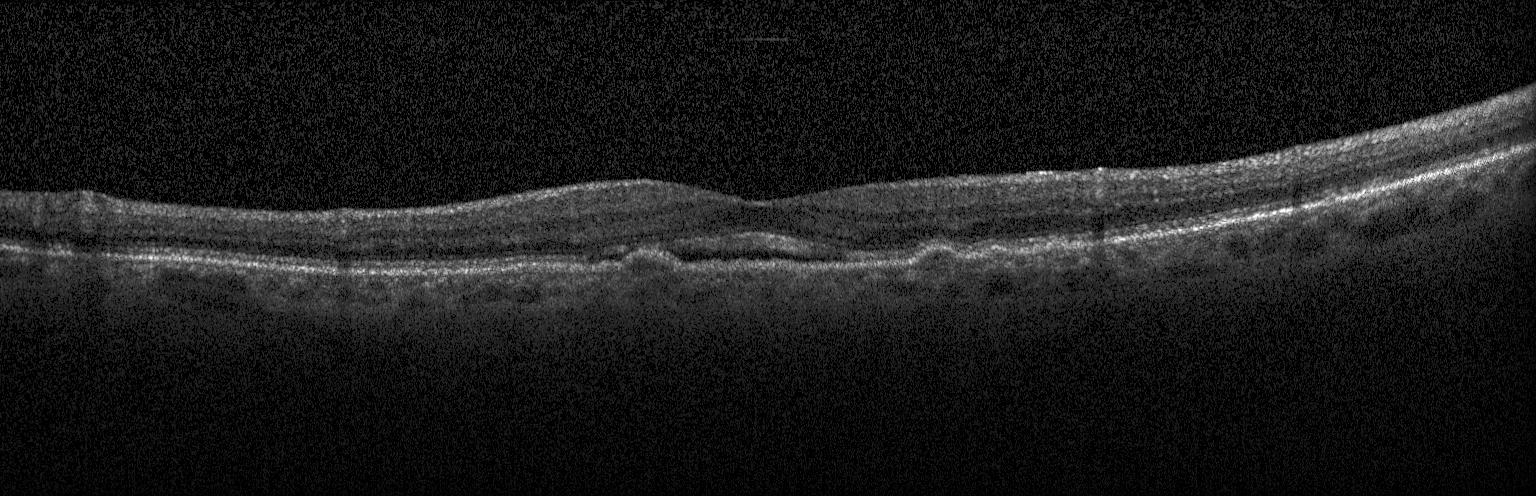
Acquired on a Heidelberg Spectralis · OCT line scan — Macular OCT: choroidal neovascularization (CNV).